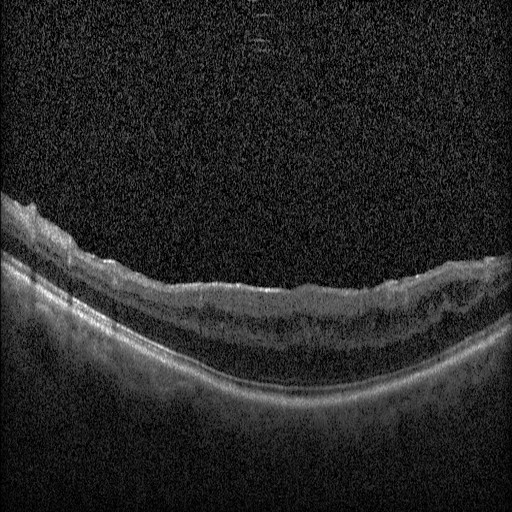
Horizontal scan through the fovea. OCT line scan. Heidelberg Spectralis
Diagnosis: diabetic macular edema.